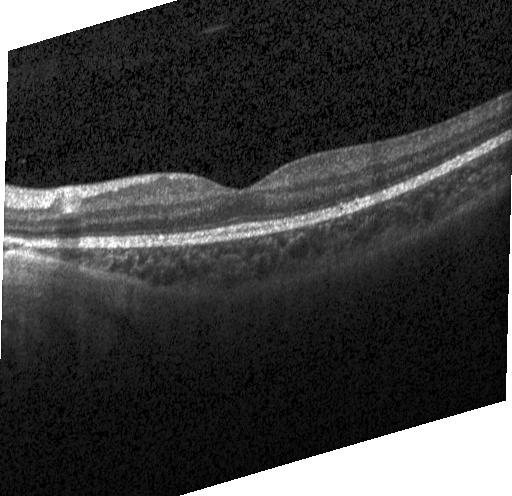 Optical coherence tomography scan, centered on the fovea. Diagnosis: neither CNV, DME, nor drusen.